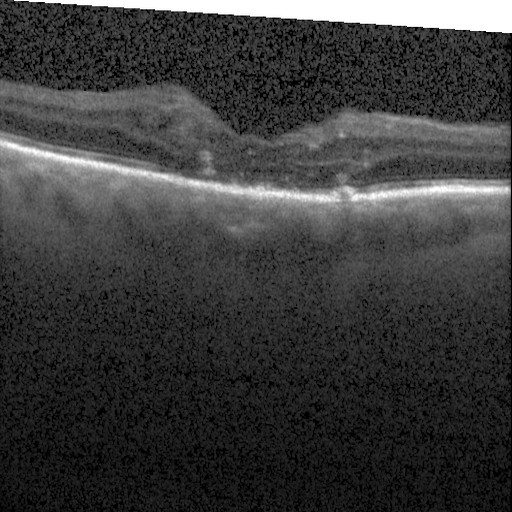
Retinal OCT cross-section
The scan shows diabetic macular edema.